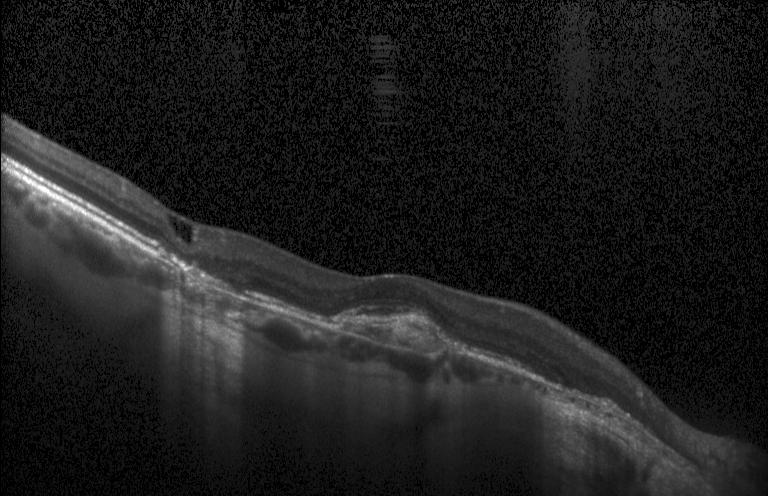
Retinal OCT B-scan
Finding: a choroidal neovascular membrane.